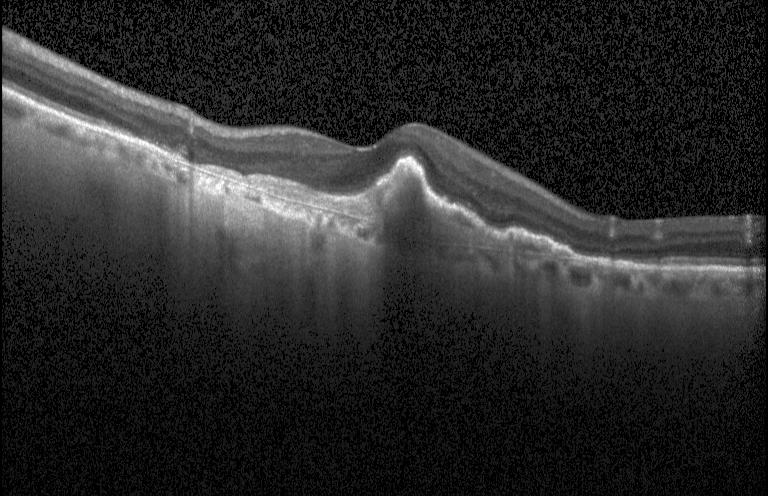

SD-OCT · acquired on a Heidelberg Spectralis · optical coherence tomography scan.
Diagnosis: choroidal neovascularization (CNV).